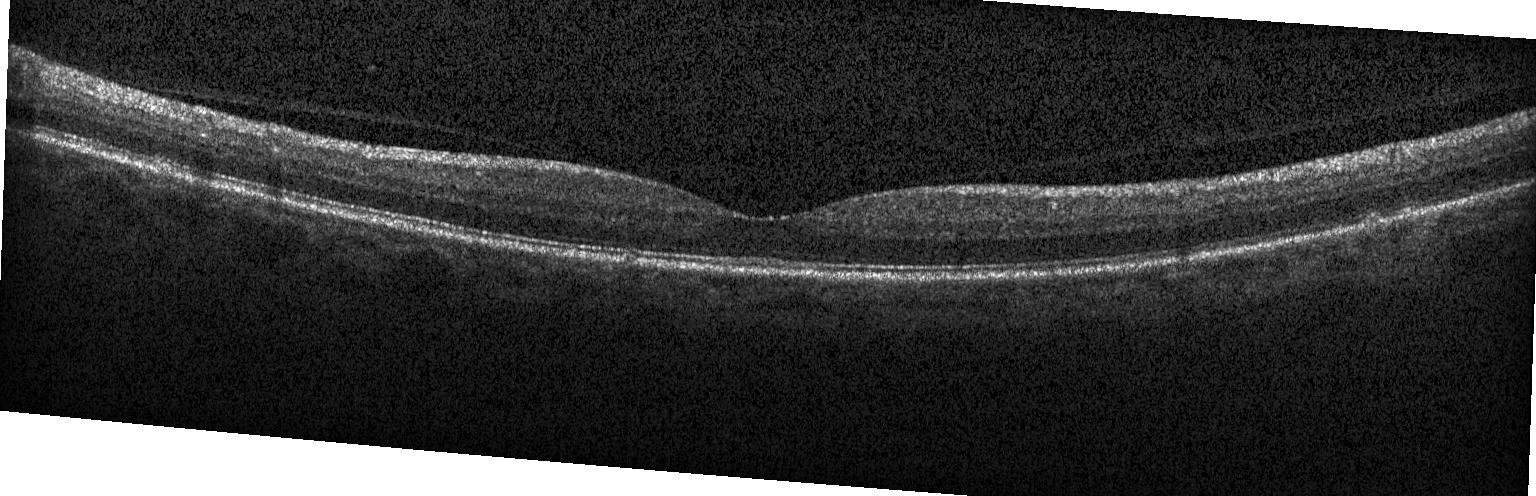
OCT finding: neither choroidal neovascularization, diabetic macular edema, nor drusen.